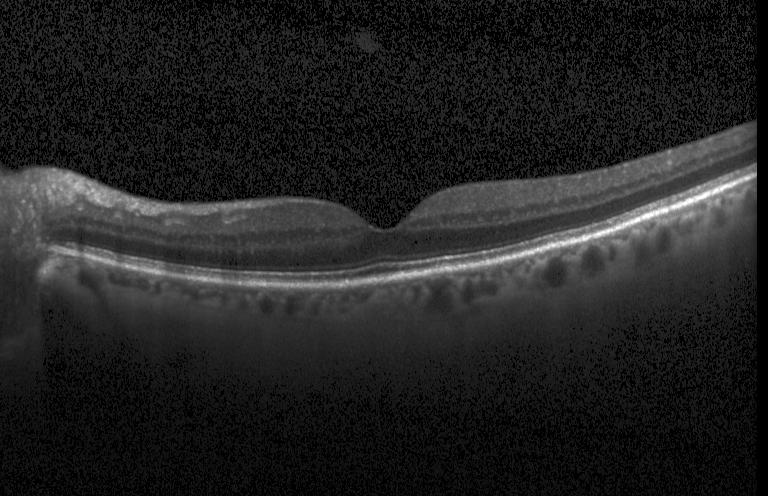 Spectral-domain optical coherence tomography. Fovea-centered. Retinal OCT B-scan.
Diagnosis: neither choroidal neovascularization, diabetic macular edema, nor drusen.